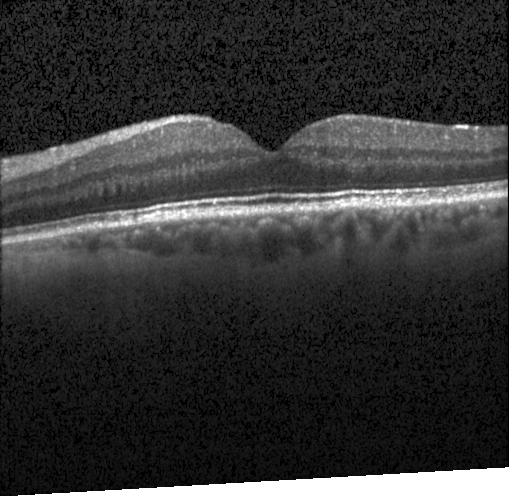

OCT line scan, centered on the fovea, instrument: Heidelberg Spectralis, SD-OCT
Macular OCT: neither choroidal neovascularization, diabetic macular edema, nor drusen.